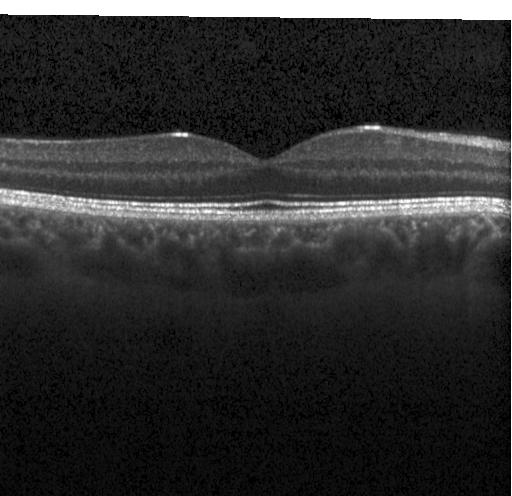
Spectral-domain OCT B-scan: no CNV, DME, or drusen.